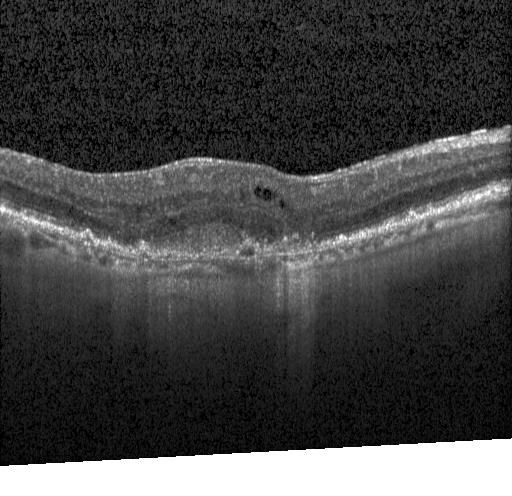 This B-scan demonstrates a choroidal neovascular membrane.